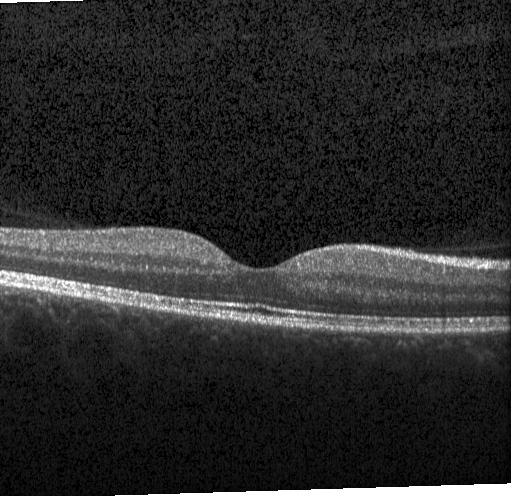 Macular OCT: neither choroidal neovascularization, diabetic macular edema, nor drusen.